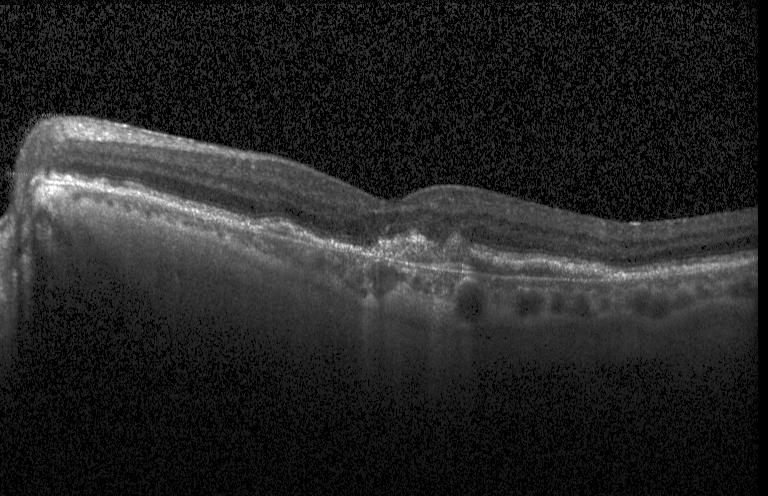 Retinal OCT cross-section. Instrument: Heidelberg Spectralis. Through the macula
Finding: choroidal neovascularization.